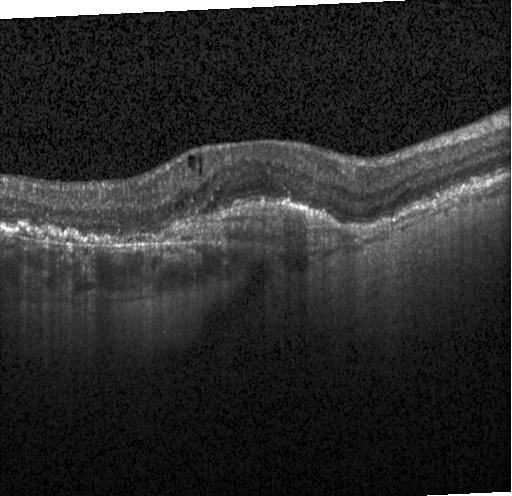
Acquired on a Heidelberg Spectralis. OCT B-scan. Spectral-domain OCT. Assessment: choroidal neovascularization.